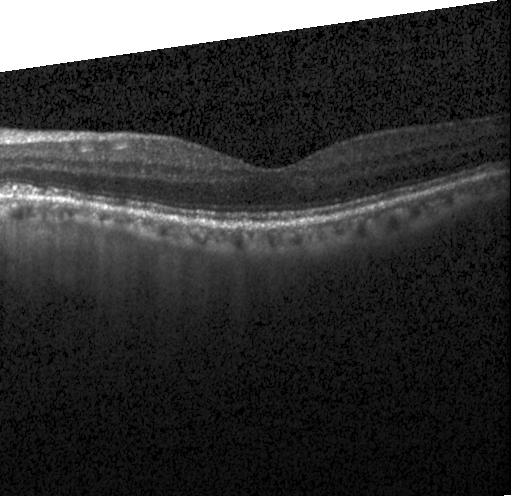
Heidelberg Spectralis; spectral-domain optical coherence tomography; optical coherence tomography scan; through the macula.
Diagnosis: neither choroidal neovascularization, diabetic macular edema, nor drusen.